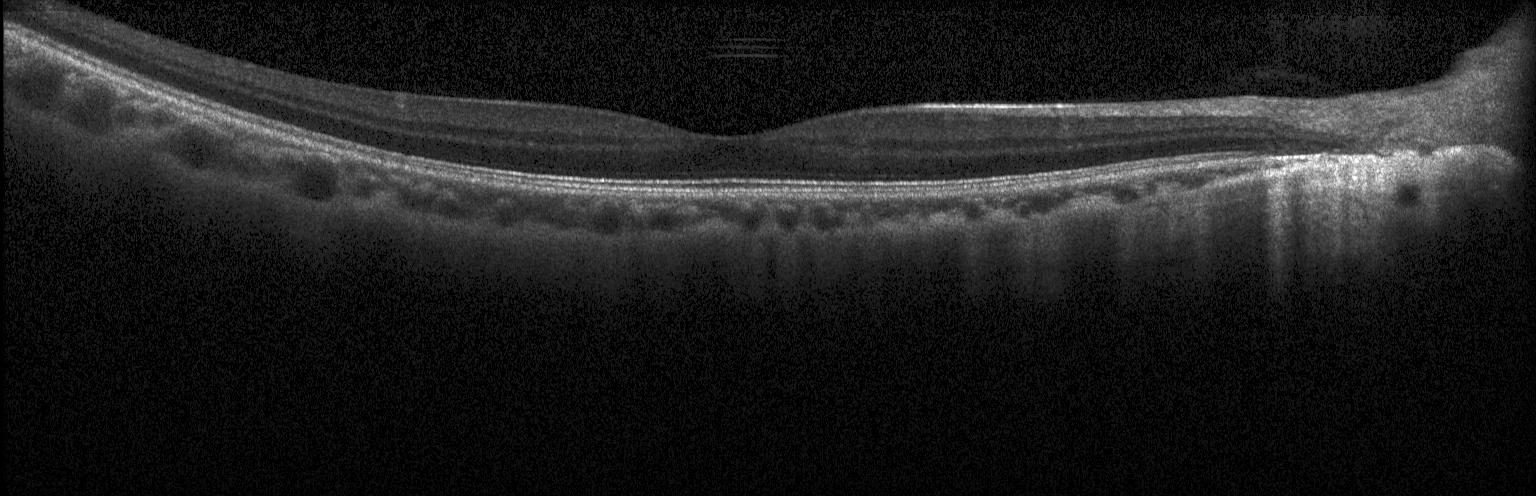

Optical coherence tomography B-scan; spectral-domain OCT; Heidelberg Spectralis
Impression: neither CNV, DME, nor drusen.